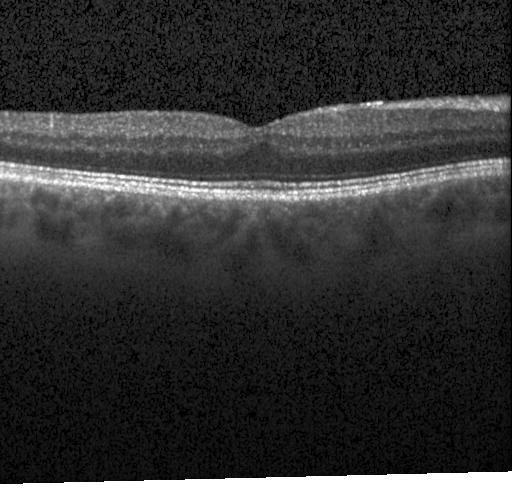

Optical coherence tomography scan. Diagnosis: no evidence of choroidal neovascularization, diabetic macular edema, or drusen.